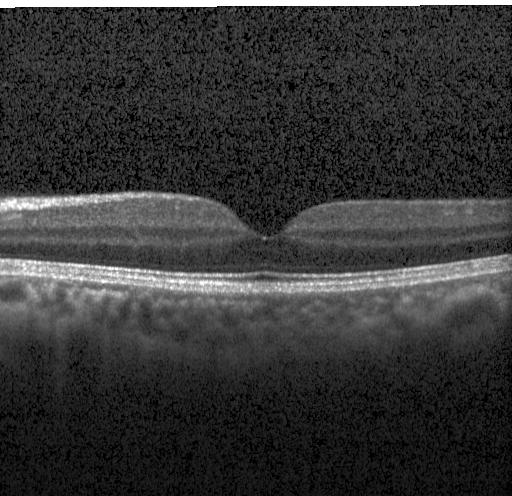

Finding: no CNV, no DME, and no drusen.